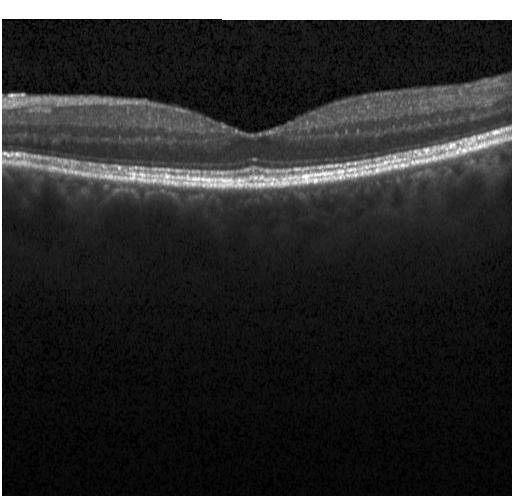

Retinal OCT B-scan
The scan shows neither choroidal neovascularization, diabetic macular edema, nor drusen.